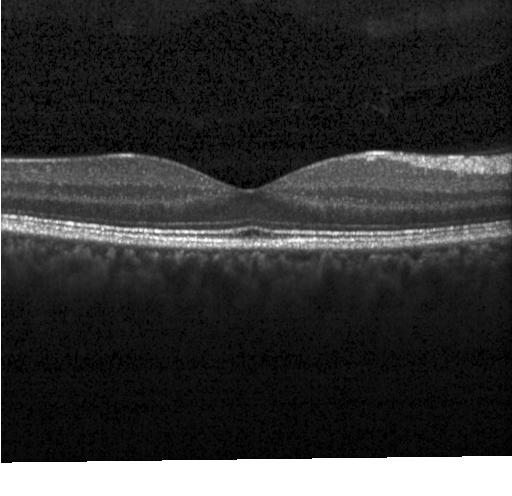
Horizontal scan through the fovea. Heidelberg Spectralis. OCT line scan. SD-OCT — Impression: no choroidal neovascularization, no diabetic macular edema, and no drusen.